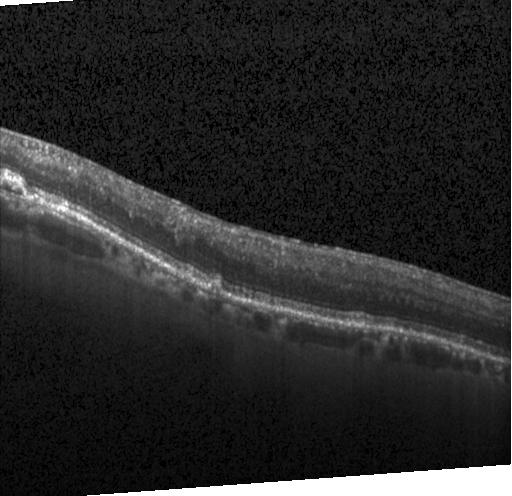 Acquired on a Heidelberg Spectralis. SD-OCT. Centered on the fovea. OCT B-scan. Diagnosis: choroidal neovascularization (CNV).